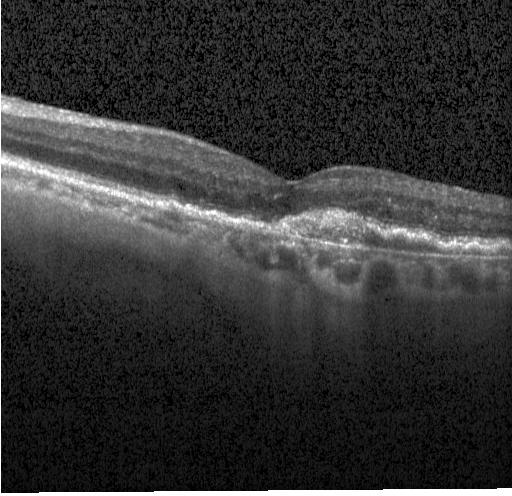
OCT B-scan · through the macula · instrument: Heidelberg Spectralis.
Finding: a choroidal neovascular membrane.